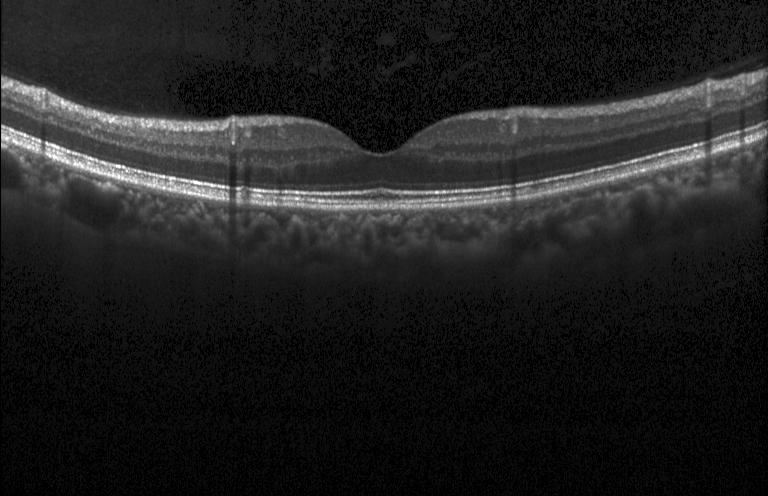
Heidelberg Spectralis · through the macula · SD-OCT · optical coherence tomography scan — The scan shows neither CNV, DME, nor drusen.